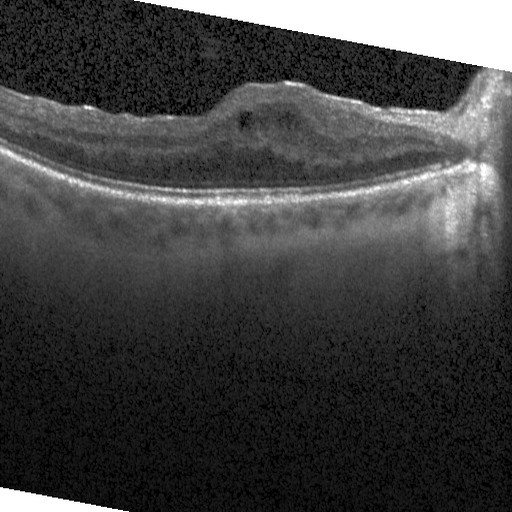 OCT finding: diabetic macular edema (DME).